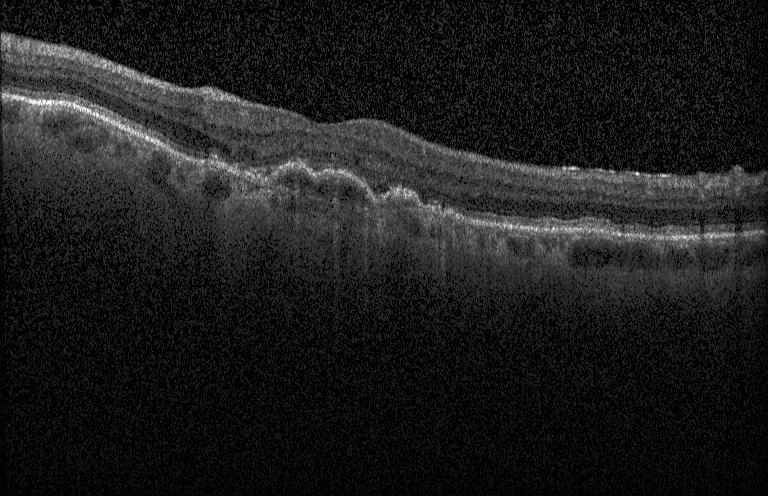
Diagnosis: CNV.